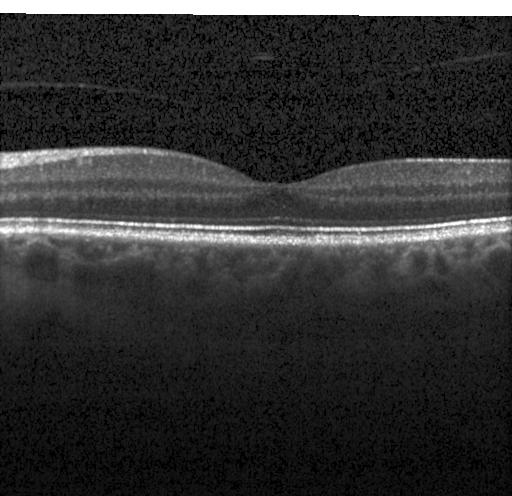

Heidelberg Spectralis · retinal OCT B-scan · through the macula · spectral-domain OCT
This B-scan demonstrates no CNV, DME, or drusen.